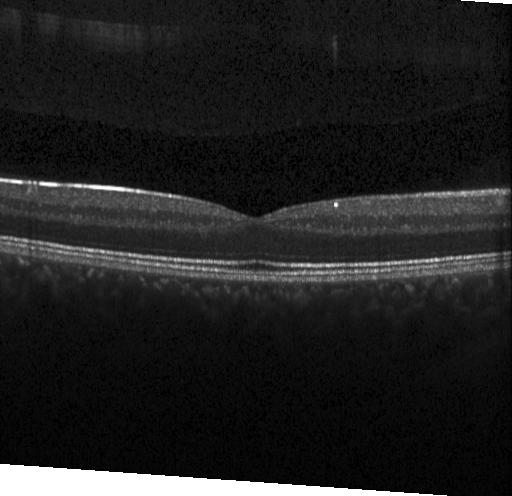 Dx: neither choroidal neovascularization, diabetic macular edema, nor drusen.